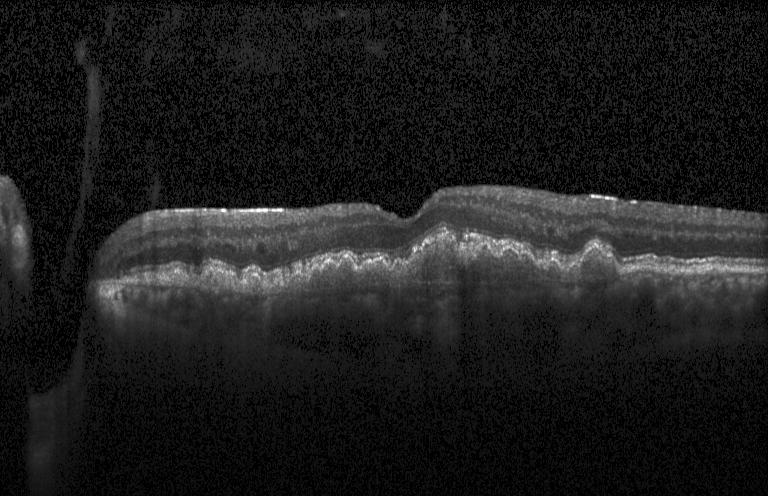 Diagnosis: CNV.